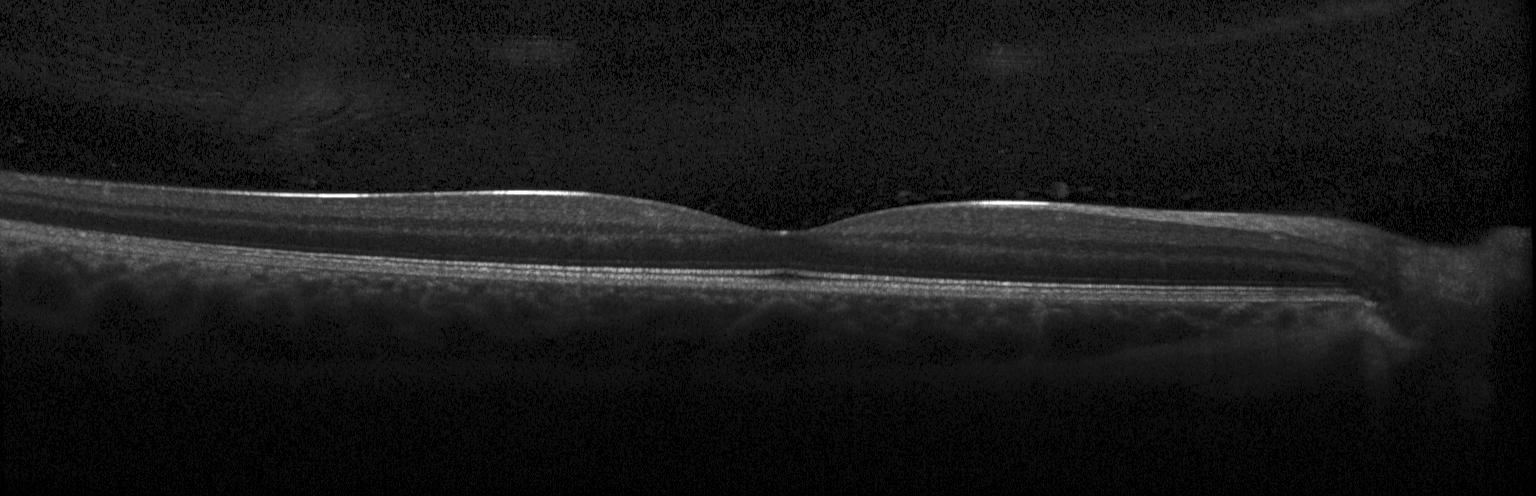
No evidence of choroidal neovascularization, diabetic macular edema, or drusen.